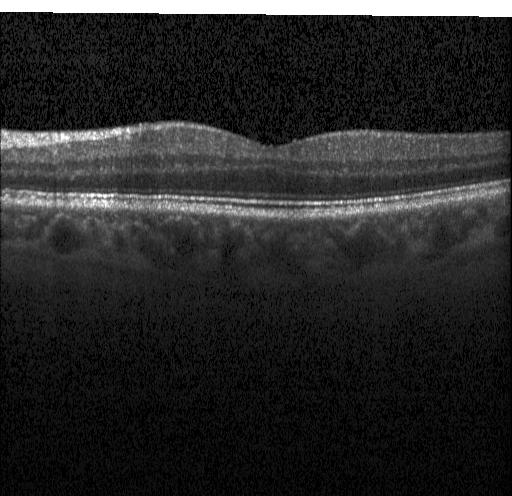 OCT B-scan. Instrument: Heidelberg Spectralis. Through the macula. Finding: no evidence of CNV, DME, or drusen.